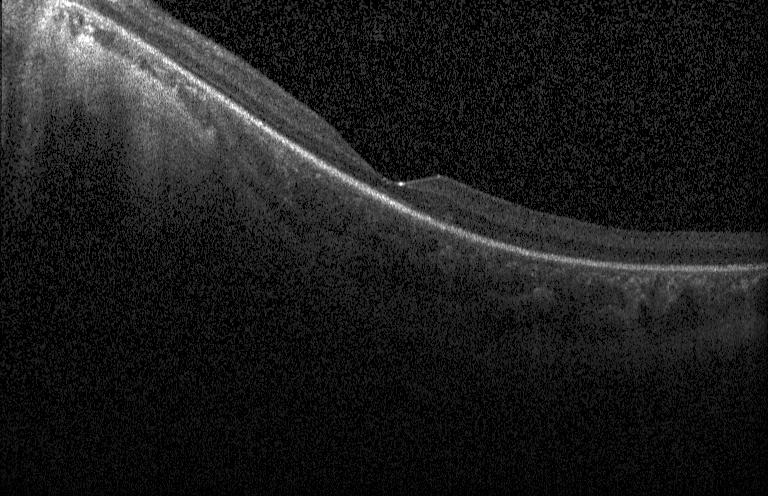
The scan shows no CNV, DME, or drusen.